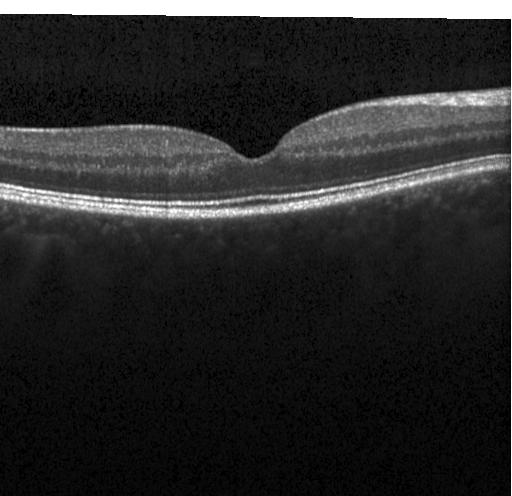
OCT line scan — Finding: no choroidal neovascularization, diabetic macular edema, or drusen.